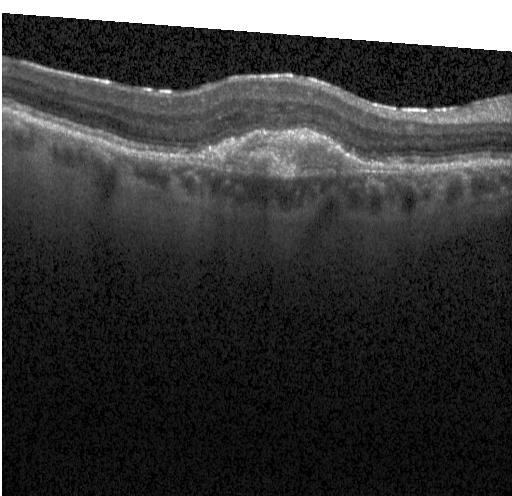 OCT B-scan.
OCT finding: a choroidal neovascular membrane.